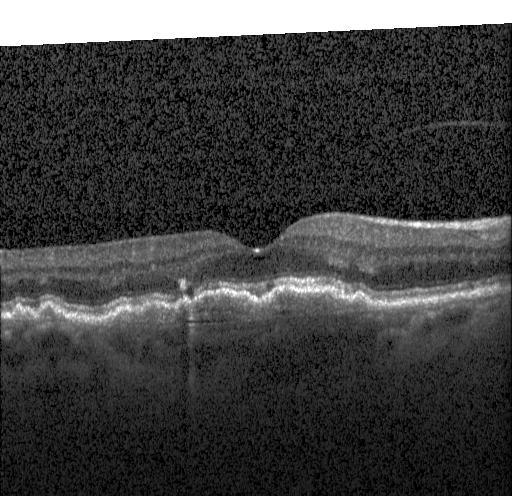 Heidelberg Spectralis. Retinal OCT cross-section — A choroidal neovascular membrane.